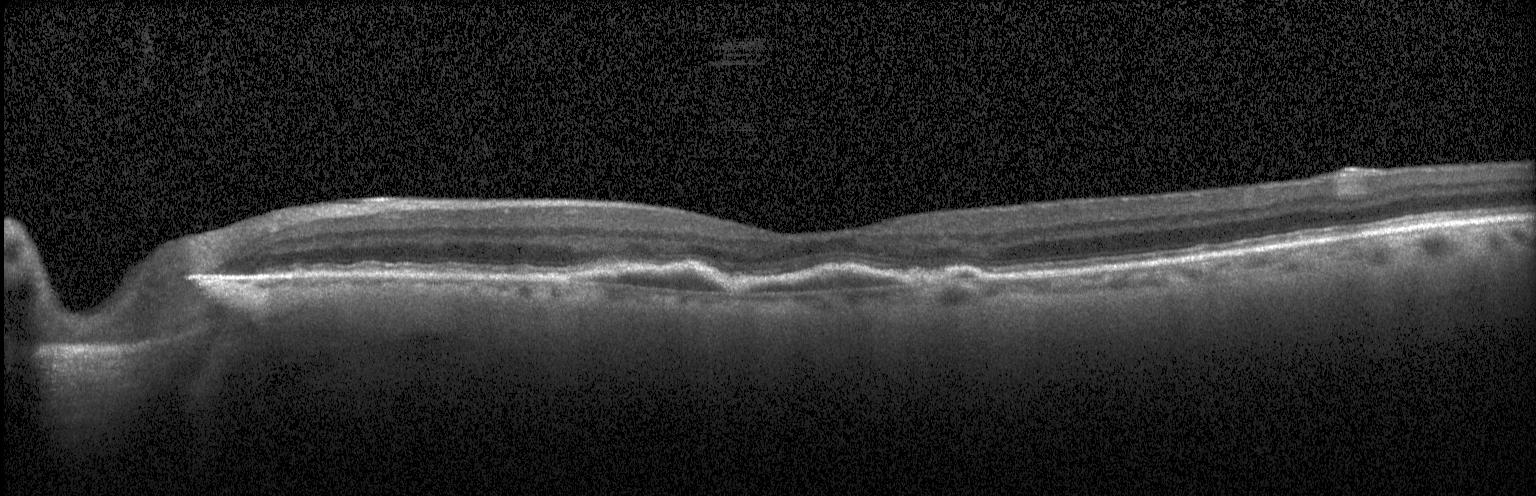
OCT line scan; through the macula
Impression: CNV.